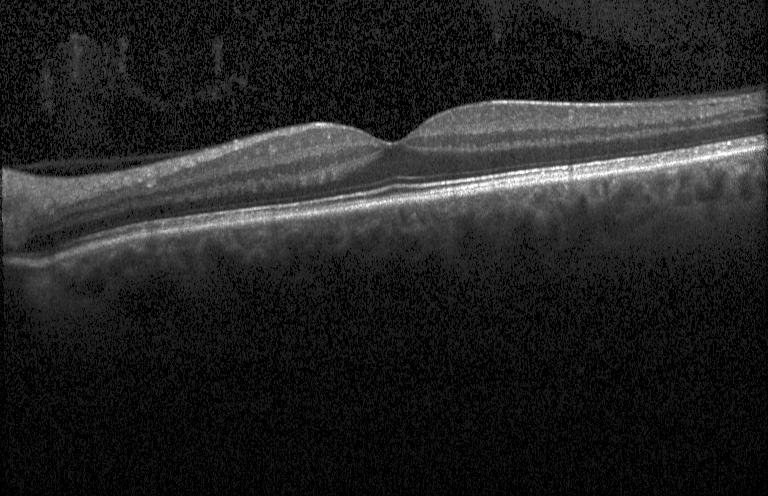

No evidence of choroidal neovascularization, diabetic macular edema, or drusen.